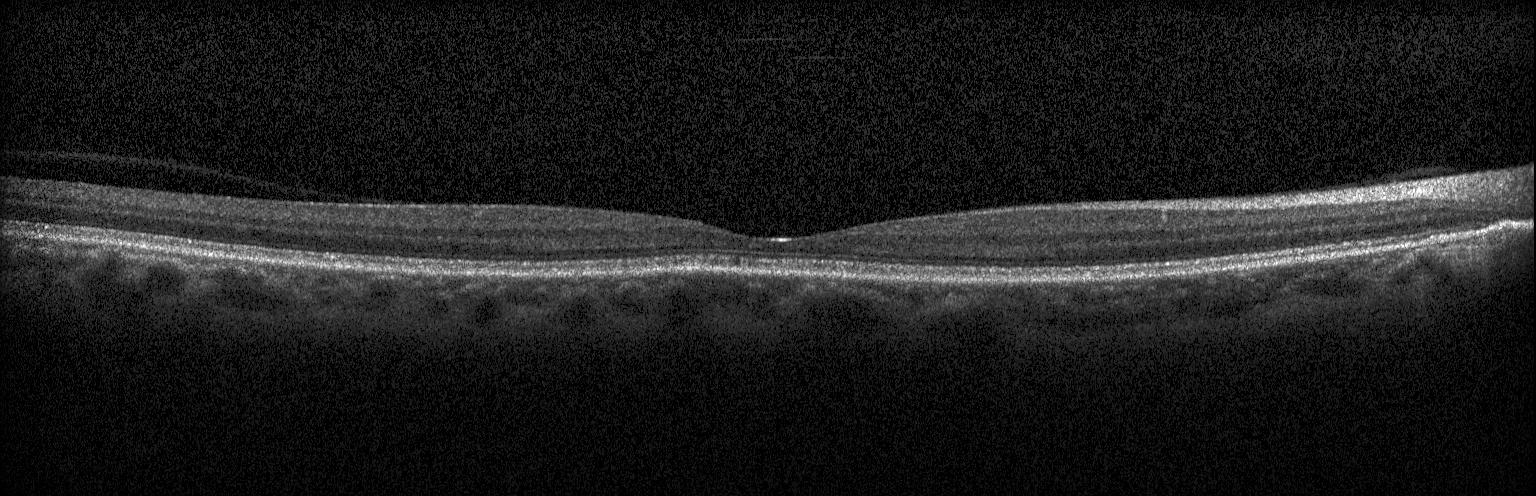 Optical coherence tomography scan; SD-OCT — Dx: no CNV, DME, or drusen.